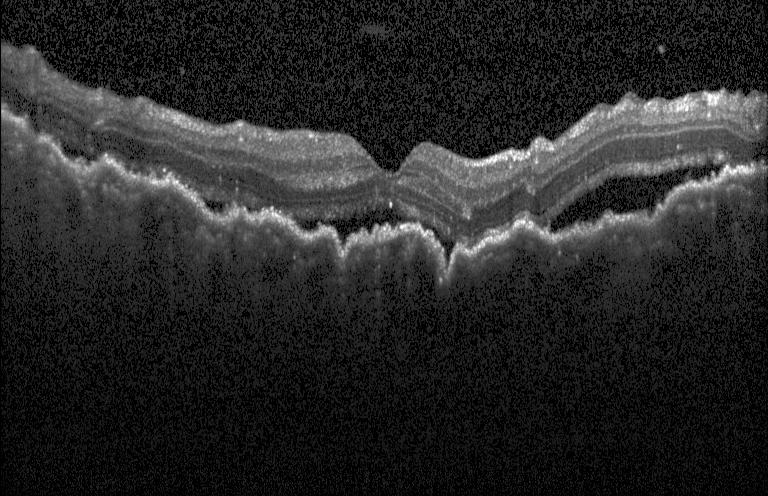

OCT finding: choroidal neovascularization (CNV).